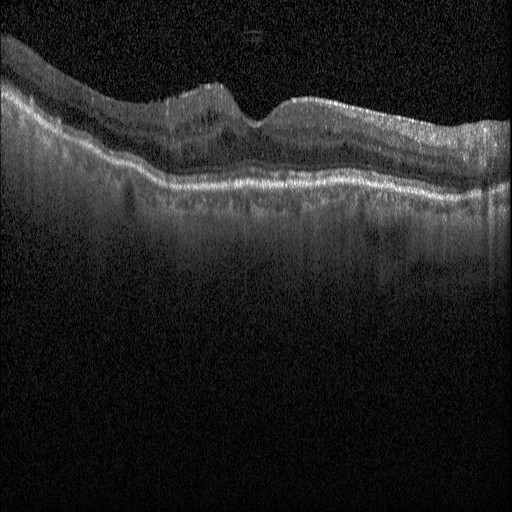

Retinal OCT B-scan. Fovea-centered.
The scan shows diabetic macular edema.